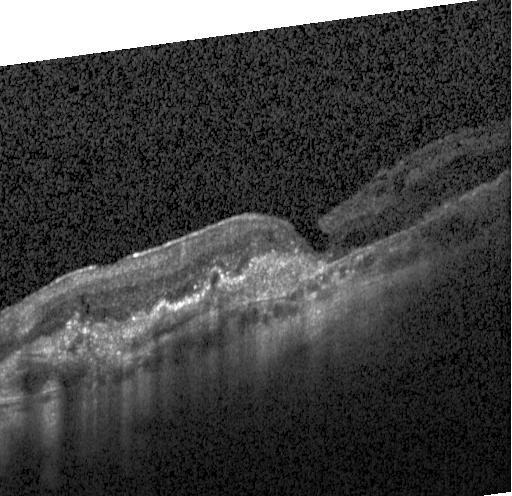

OCT line scan · through the macula · Heidelberg Spectralis OCT system — Diagnosis: a choroidal neovascular membrane.